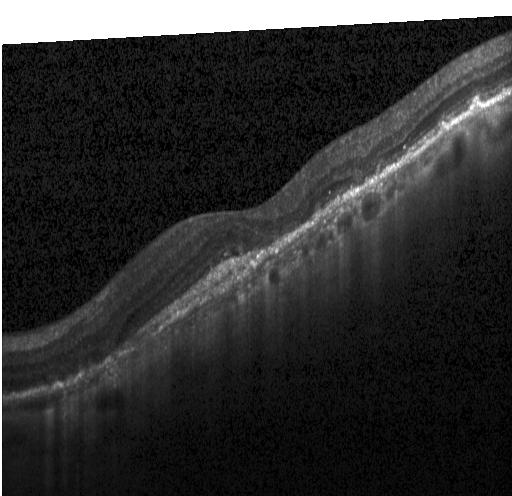 OCT line scan
The scan shows a choroidal neovascular membrane.